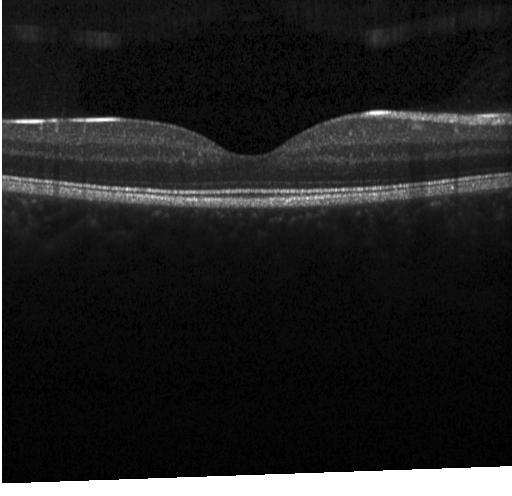
This B-scan demonstrates no CNV, DME, or drusen.